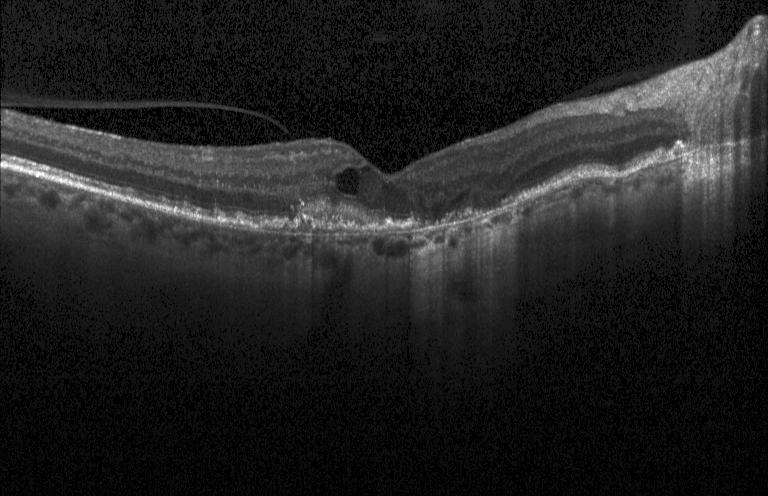
Impression: a choroidal neovascular membrane.